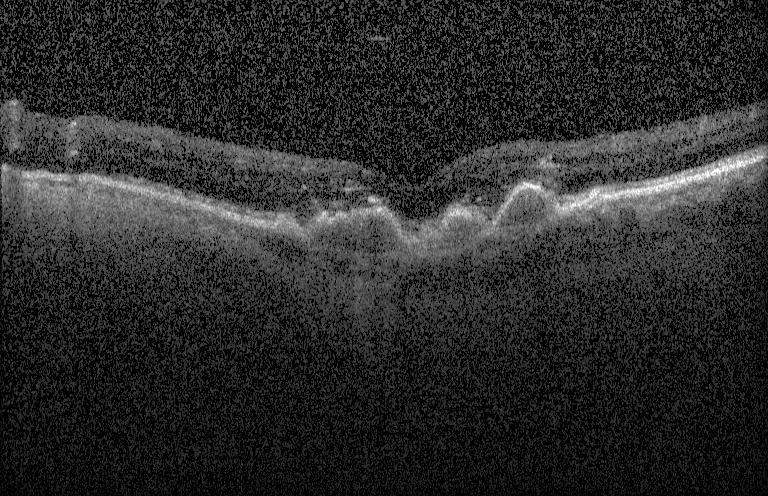

Diagnosis: a choroidal neovascular membrane.